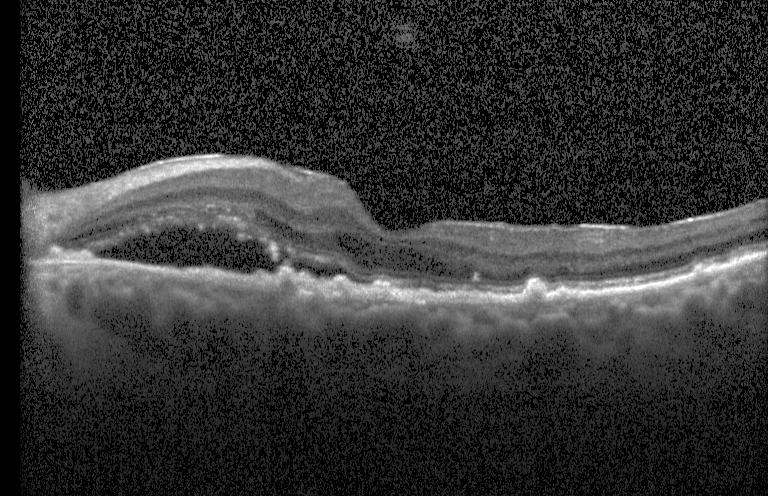

Diagnosis: a choroidal neovascular membrane.